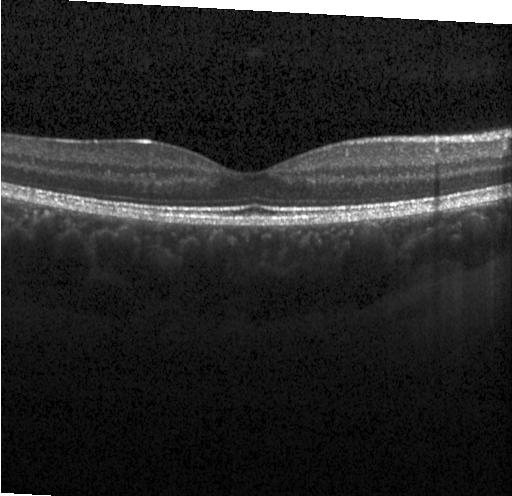

OCT finding: neither choroidal neovascularization, diabetic macular edema, nor drusen.